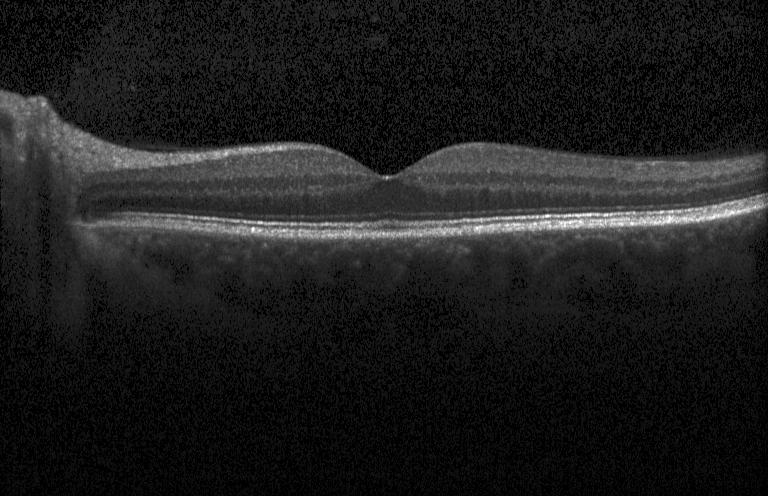 The scan shows neither choroidal neovascularization, diabetic macular edema, nor drusen.